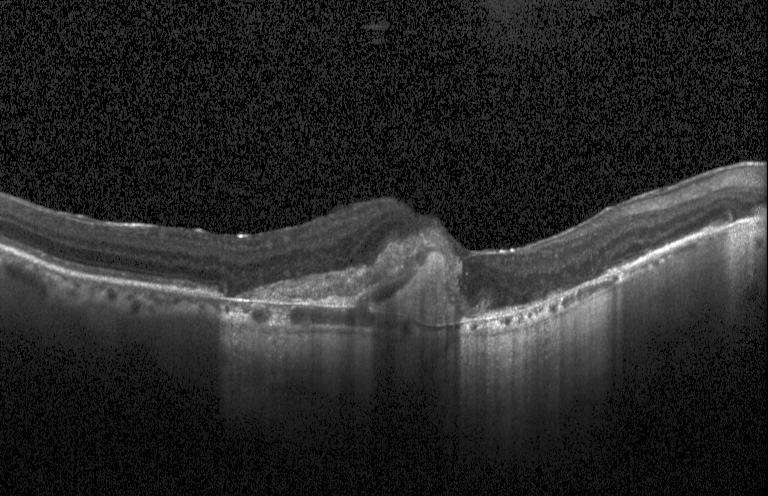 Dx: a choroidal neovascular membrane.